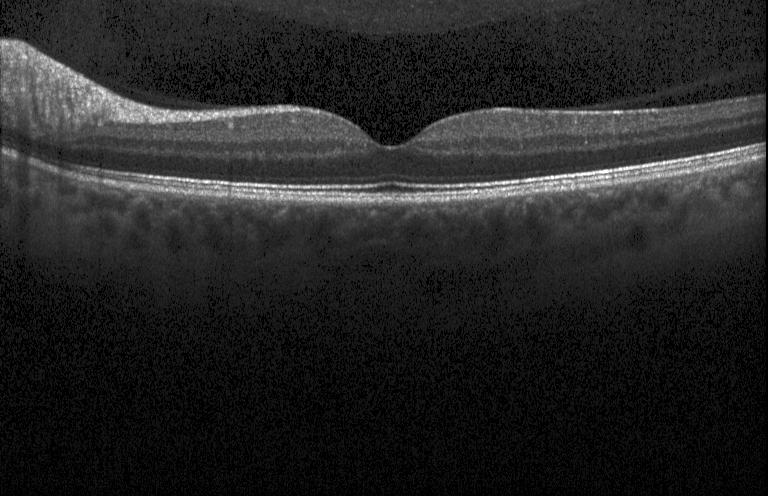

Diagnosis: neither CNV, DME, nor drusen.